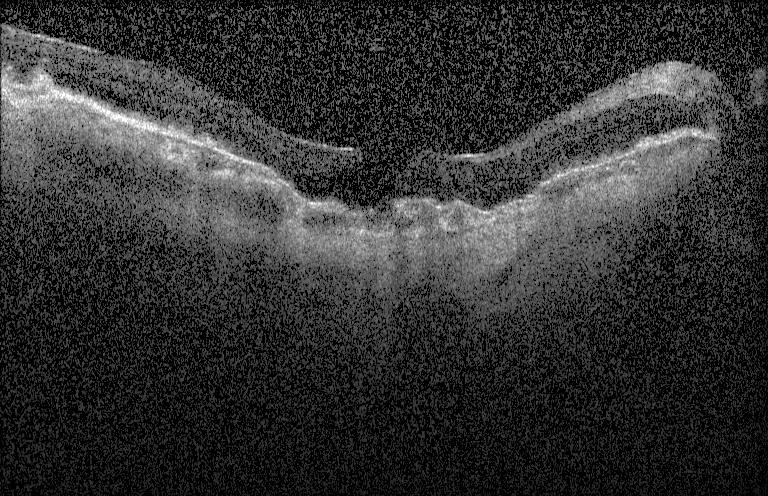 Dx: a choroidal neovascular membrane.